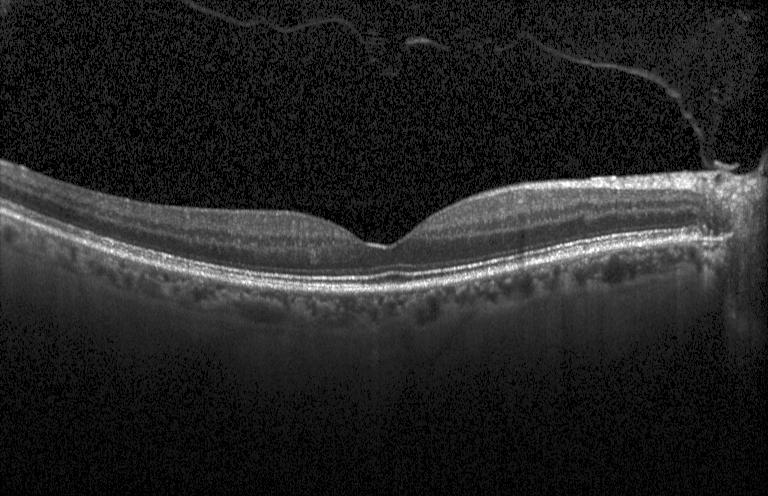
Impression: neither CNV, DME, nor drusen.